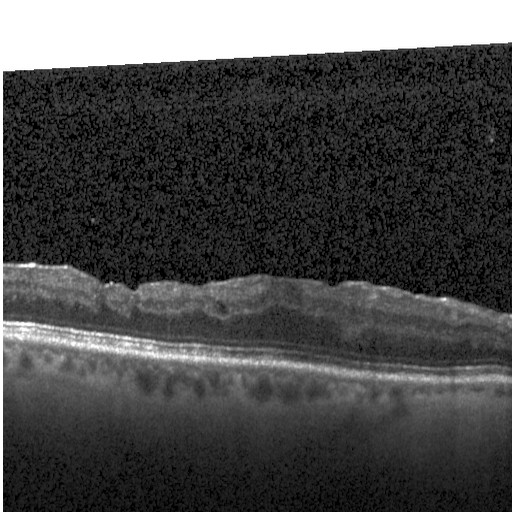 Finding: DME.